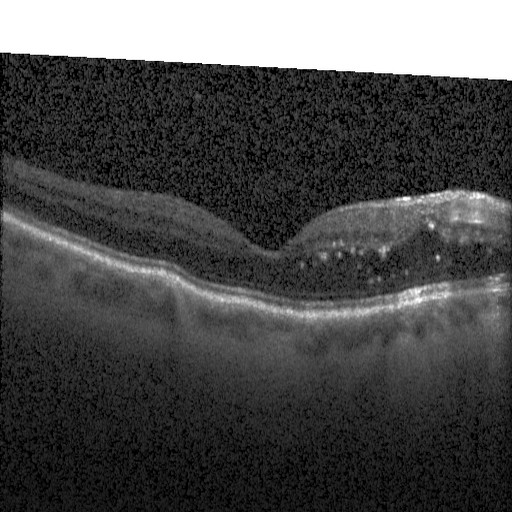 Diagnosis: DME.